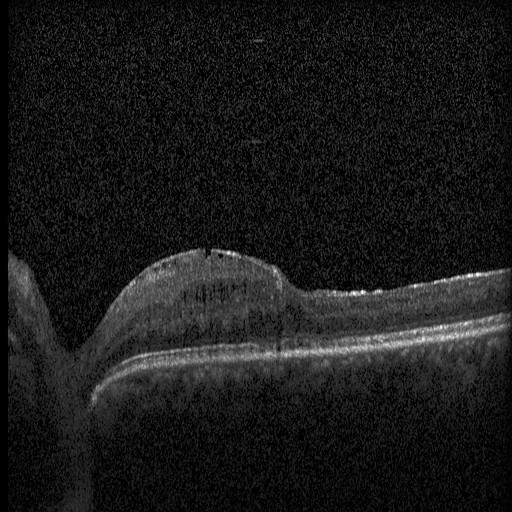 Finding: diabetic macular edema.